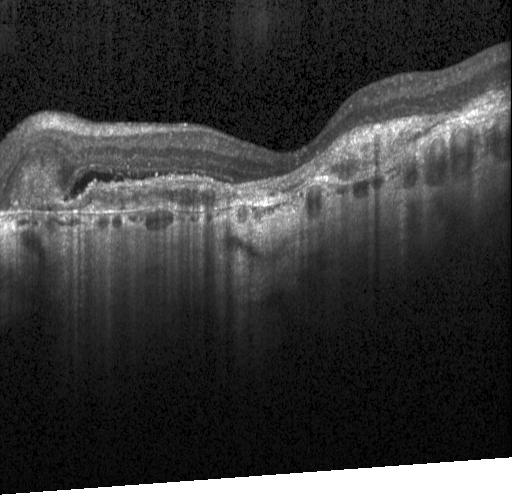

Heidelberg Spectralis, spectral-domain OCT, retinal OCT cross-section — Impression: CNV.